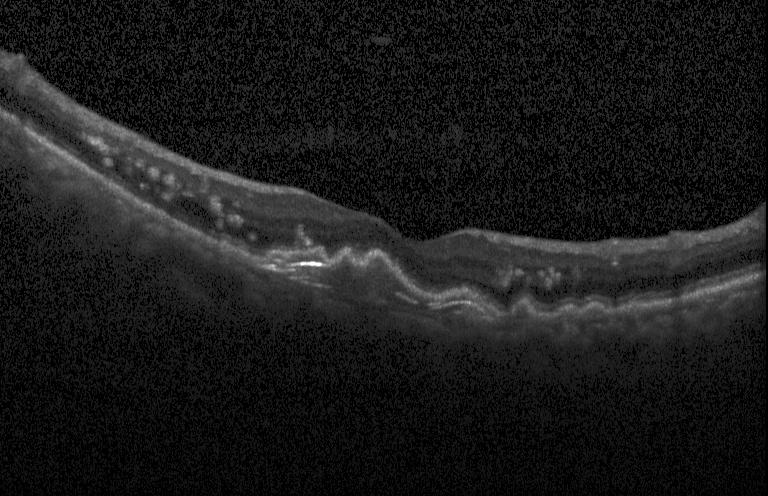 Through the macula · Heidelberg Spectralis OCT system · optical coherence tomography scan · SD-OCT.
Diagnosis: a choroidal neovascular membrane.